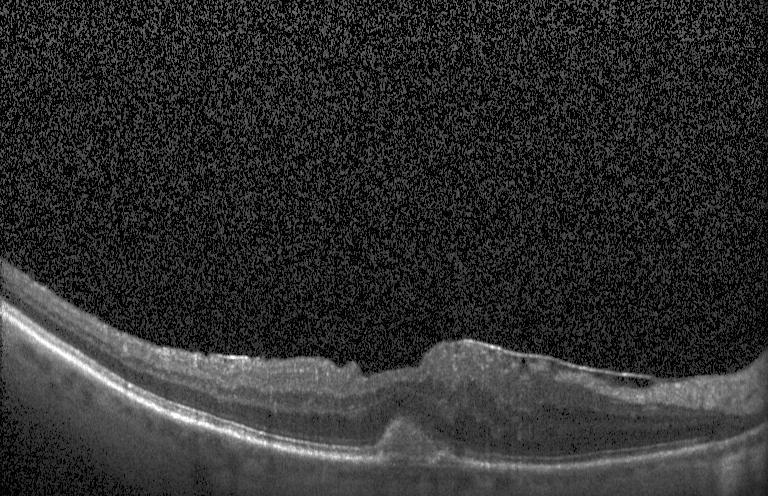 Spectral-domain optical coherence tomography · retinal OCT cross-section.
The scan shows a choroidal neovascular membrane.